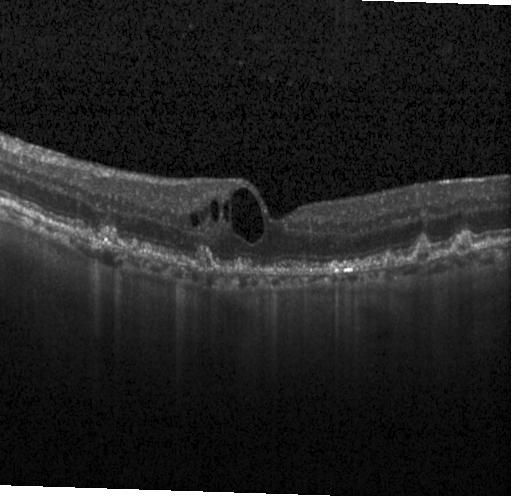

Impression: a choroidal neovascular membrane.